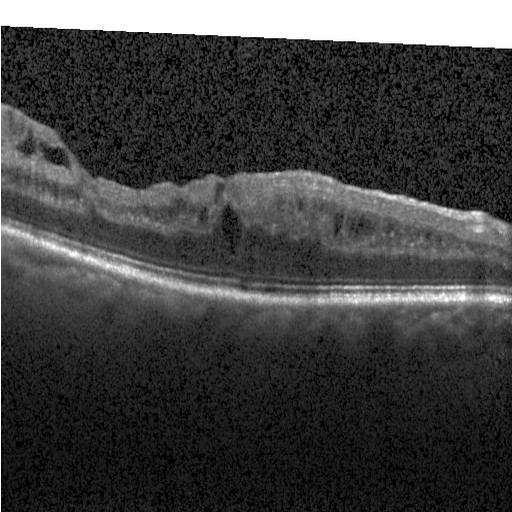 The scan shows DME.